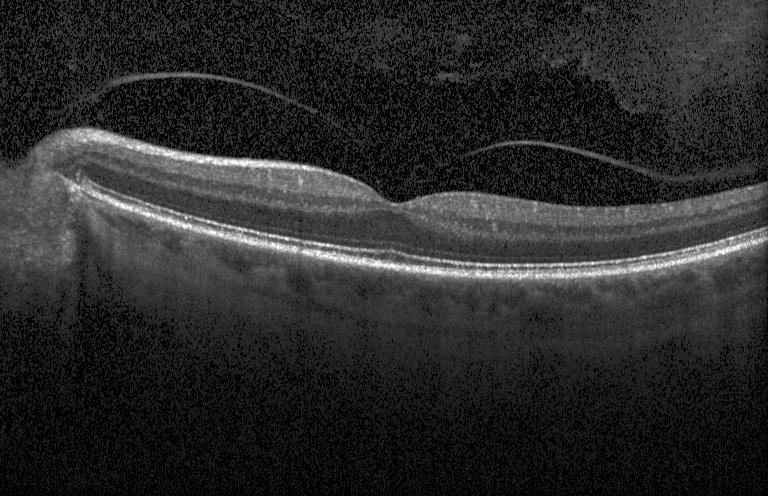 Horizontal scan through the fovea, OCT line scan.
Impression: no choroidal neovascularization, no diabetic macular edema, and no drusen.